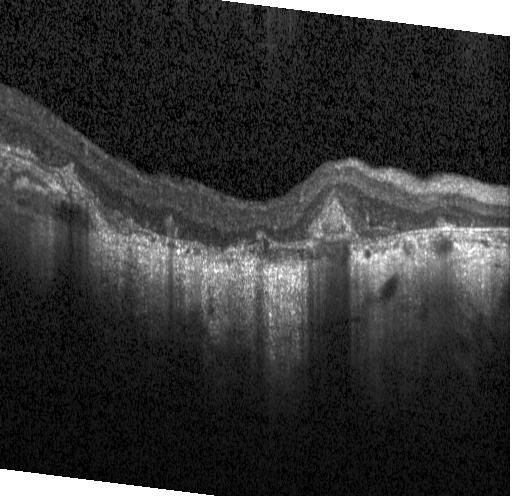 Retinal OCT B-scan.
Macular OCT: choroidal neovascularization.